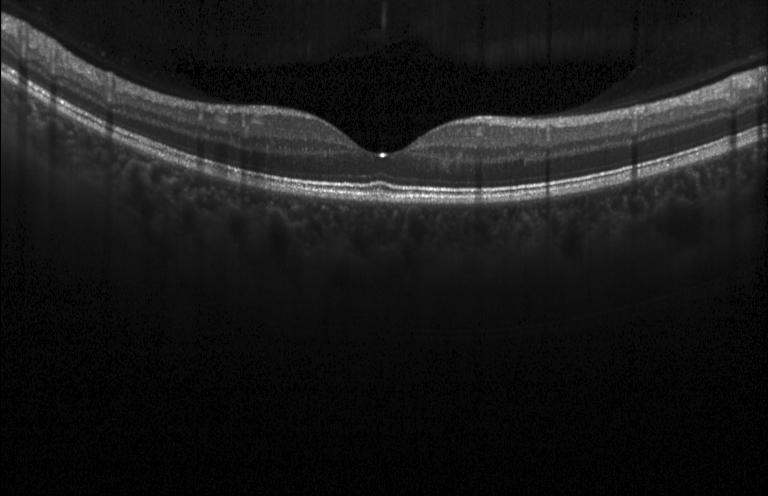
This B-scan demonstrates no choroidal neovascularization, diabetic macular edema, or drusen.